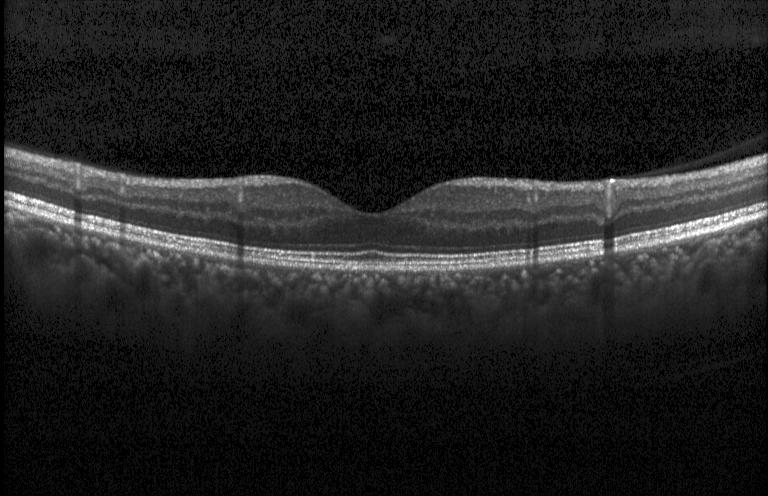
Diagnosis: neither CNV, DME, nor drusen.